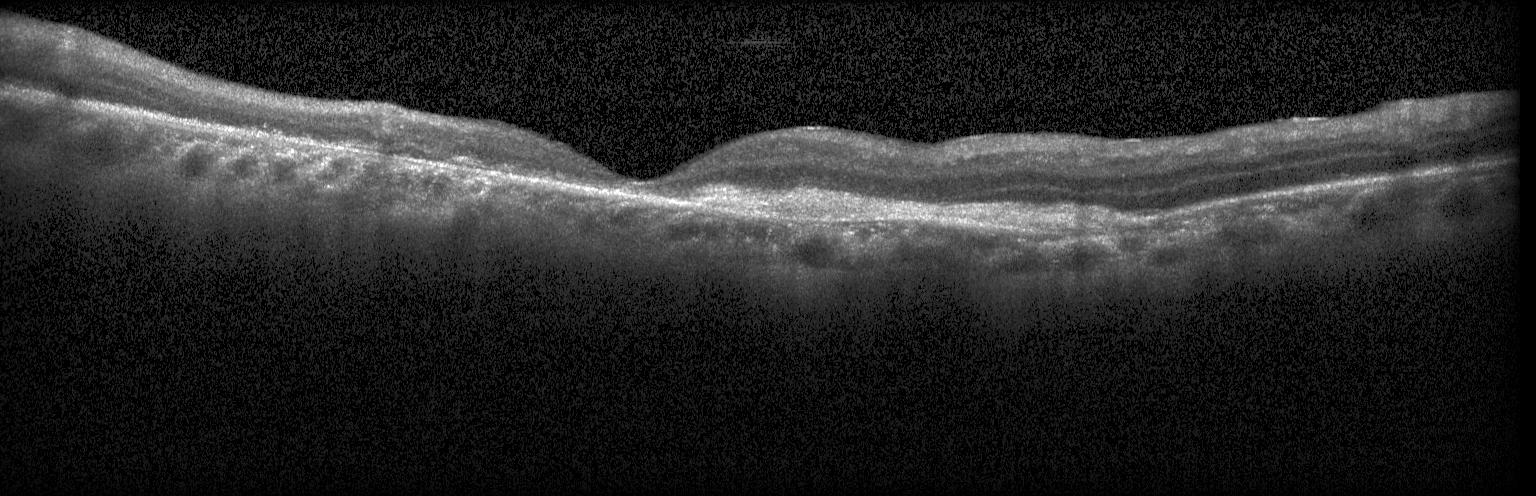
OCT scan showing a choroidal neovascular membrane.